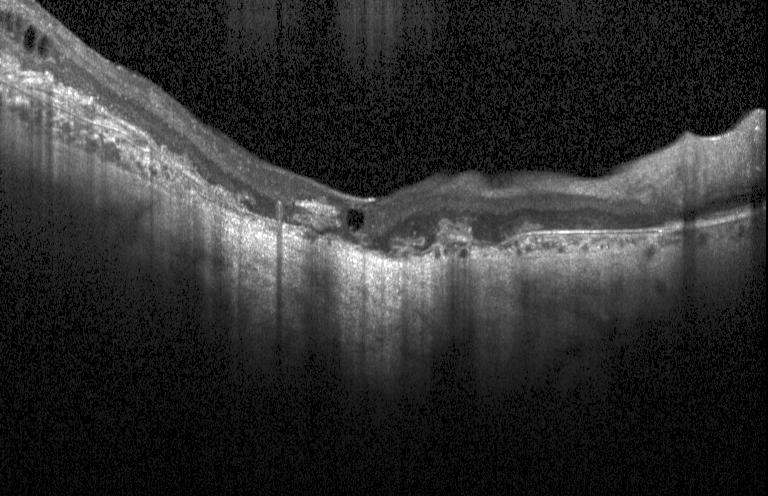

Finding: a choroidal neovascular membrane.